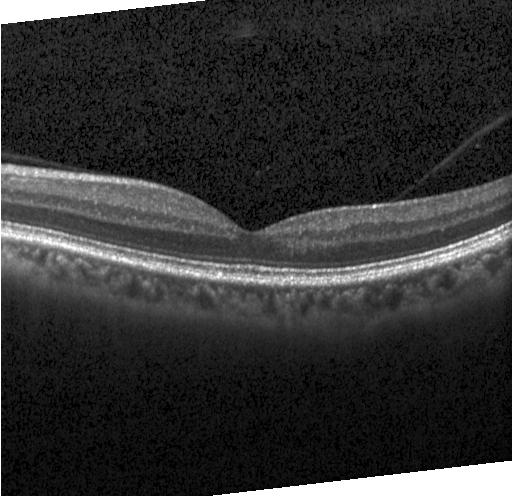 Optical coherence tomography B-scan · Heidelberg Spectralis · SD-OCT — Finding: no choroidal neovascularization, diabetic macular edema, or drusen.